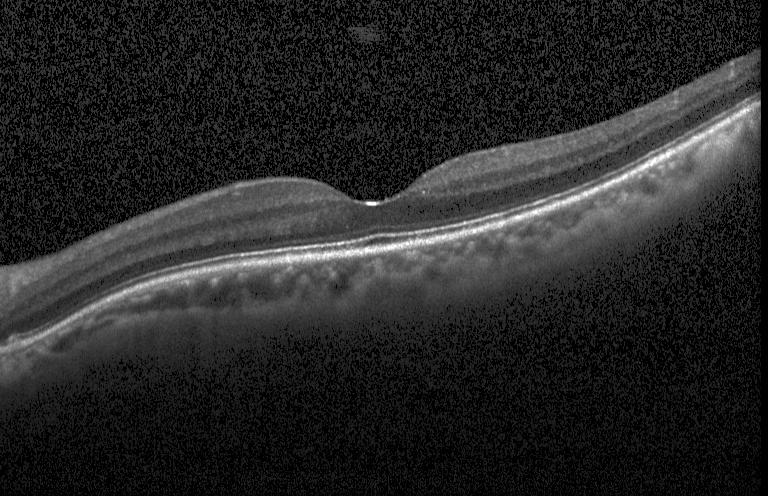

Centered on the fovea · optical coherence tomography B-scan · instrument: Heidelberg Spectralis.
The scan shows no evidence of choroidal neovascularization, diabetic macular edema, or drusen.